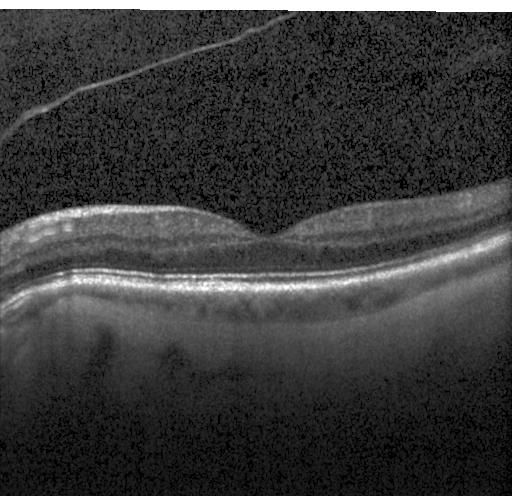 Spectral-domain OCT. Heidelberg Spectralis OCT system. Optical coherence tomography B-scan. Through the macula — The scan shows no evidence of choroidal neovascularization, diabetic macular edema, or drusen.